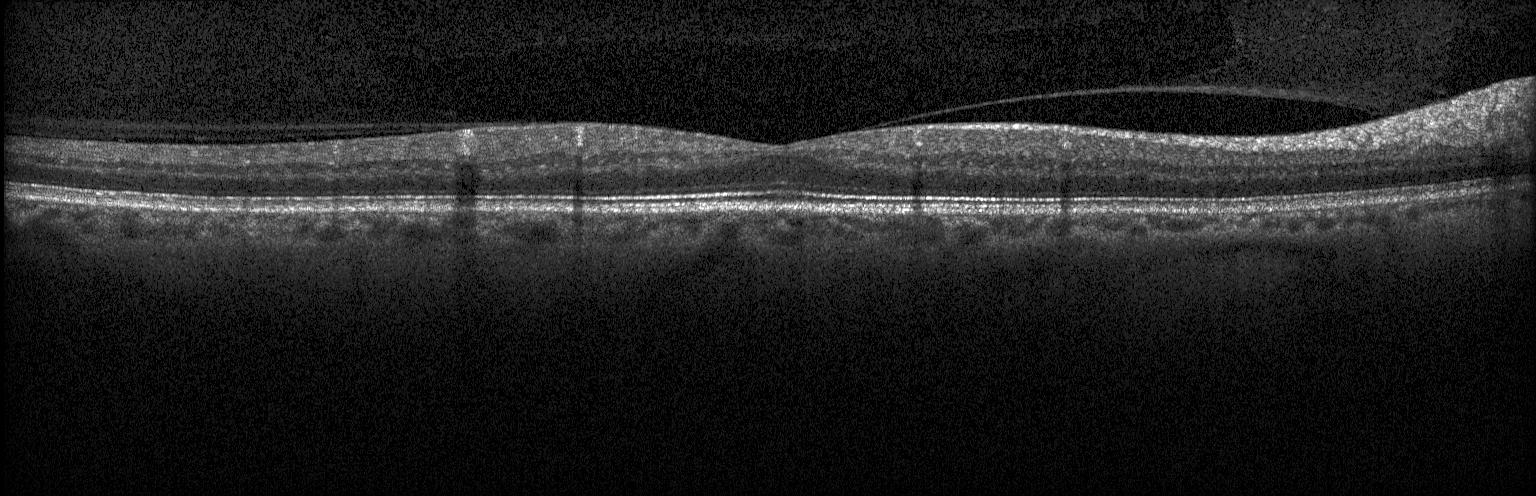
Fovea-centered · OCT line scan · acquired on a Heidelberg Spectralis · SD-OCT — Dx: no choroidal neovascularization, no diabetic macular edema, and no drusen.